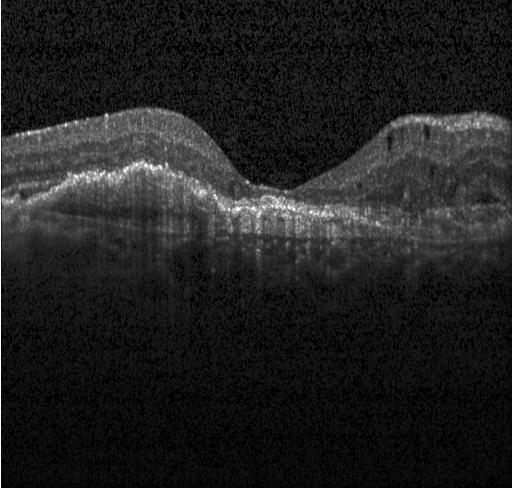

Acquired on a Heidelberg Spectralis; spectral-domain optical coherence tomography; fovea-centered; retinal OCT cross-section.
Finding: a choroidal neovascular membrane.